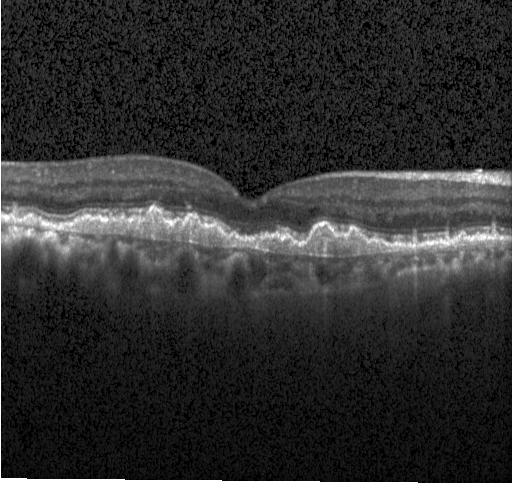

Fovea-centered; spectral-domain optical coherence tomography; OCT line scan; instrument: Heidelberg Spectralis — OCT finding: CNV.